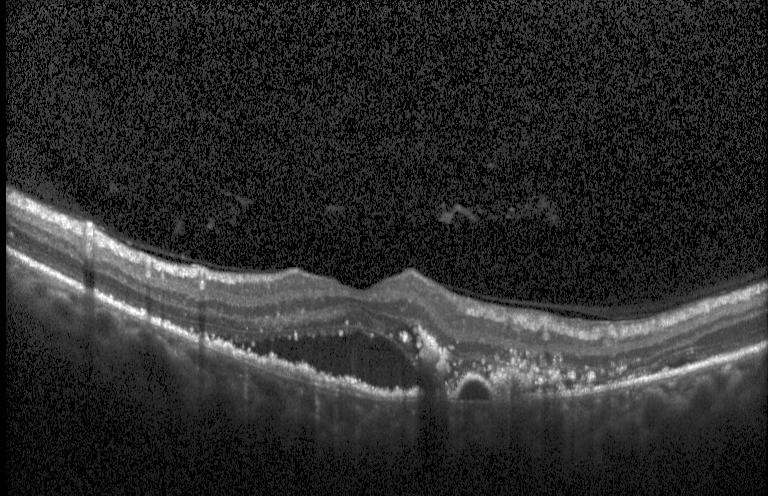 OCT line scan — Assessment: a choroidal neovascular membrane.